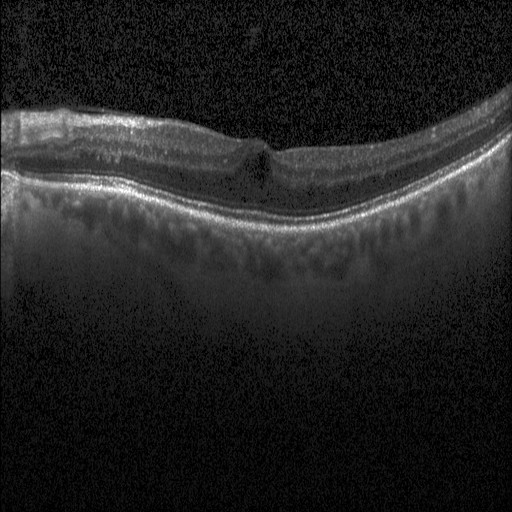 Horizontal scan through the fovea; retinal OCT cross-section; SD-OCT — OCT finding: DME.